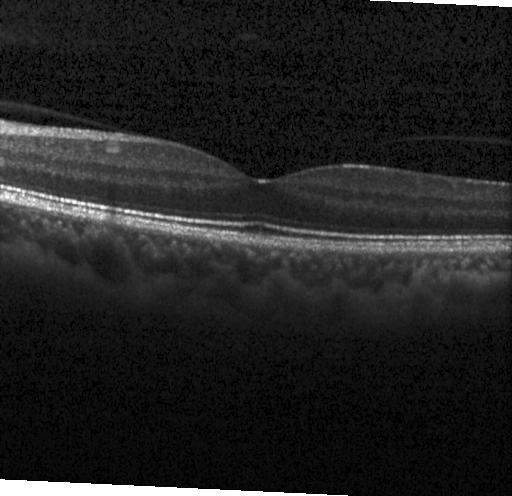

Heidelberg Spectralis OCT system, SD-OCT, optical coherence tomography B-scan.
This B-scan demonstrates no CNV, no DME, and no drusen.